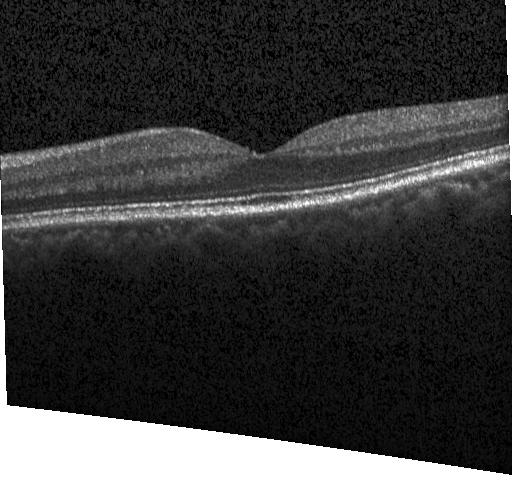

OCT finding: neither choroidal neovascularization, diabetic macular edema, nor drusen.